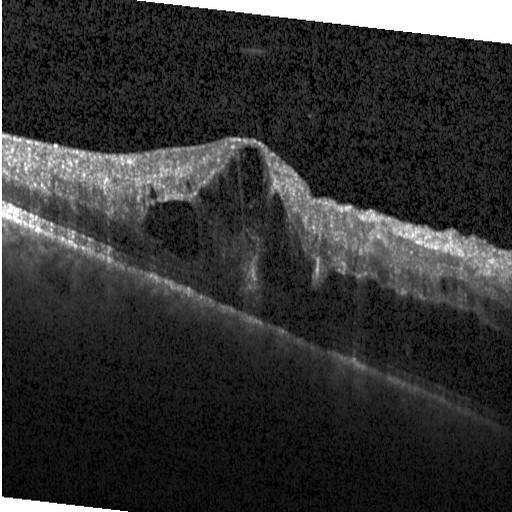
Through the macula, retinal OCT B-scan.
This B-scan demonstrates DME.